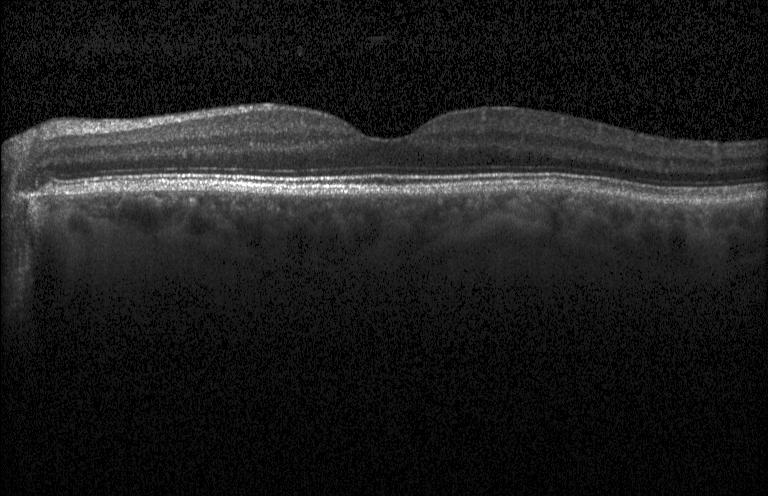
Optical coherence tomography B-scan. Heidelberg Spectralis. Finding: no choroidal neovascularization, diabetic macular edema, or drusen.